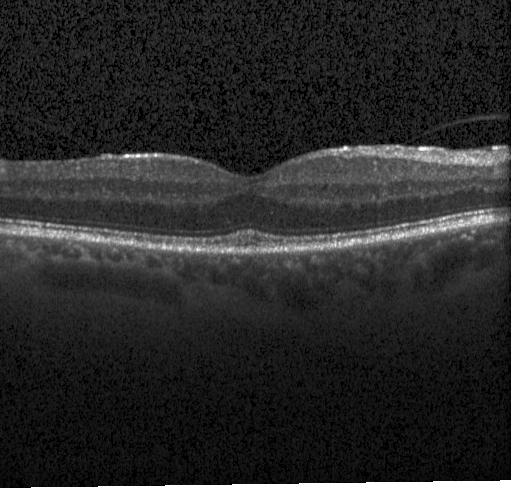 Diagnosis: no choroidal neovascularization, diabetic macular edema, or drusen.